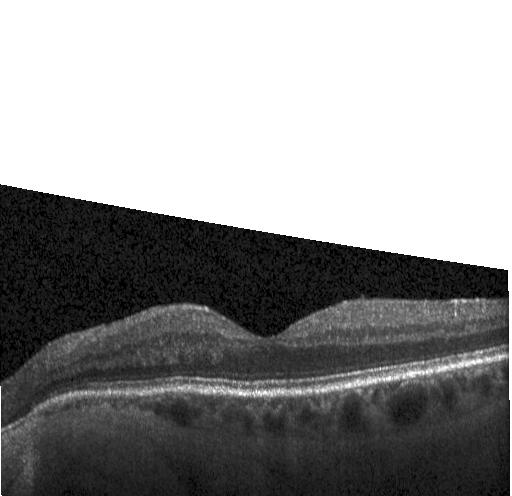 OCT B-scan · Heidelberg Spectralis OCT system
Assessment: neither choroidal neovascularization, diabetic macular edema, nor drusen.